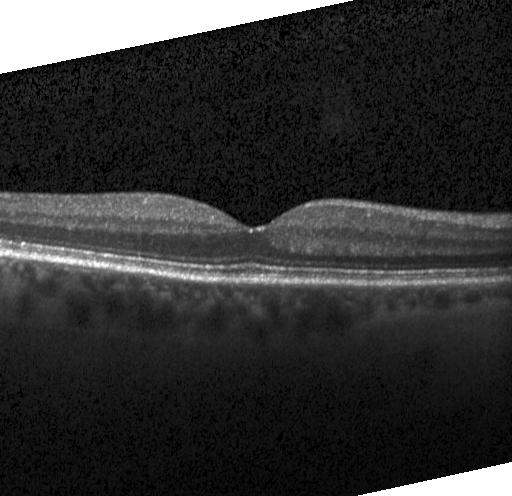
This B-scan demonstrates no evidence of choroidal neovascularization, diabetic macular edema, or drusen.